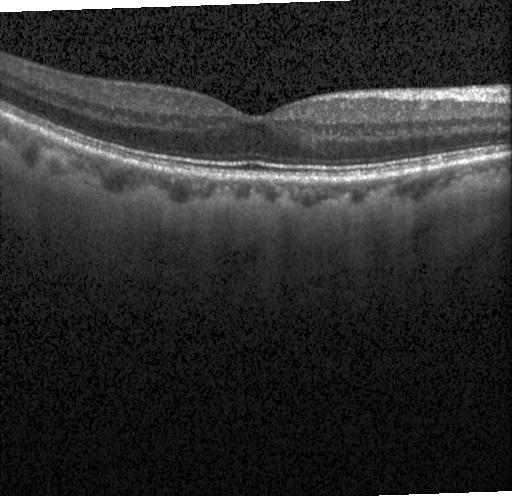

Heidelberg Spectralis; OCT line scan
Impression: neither CNV, DME, nor drusen.